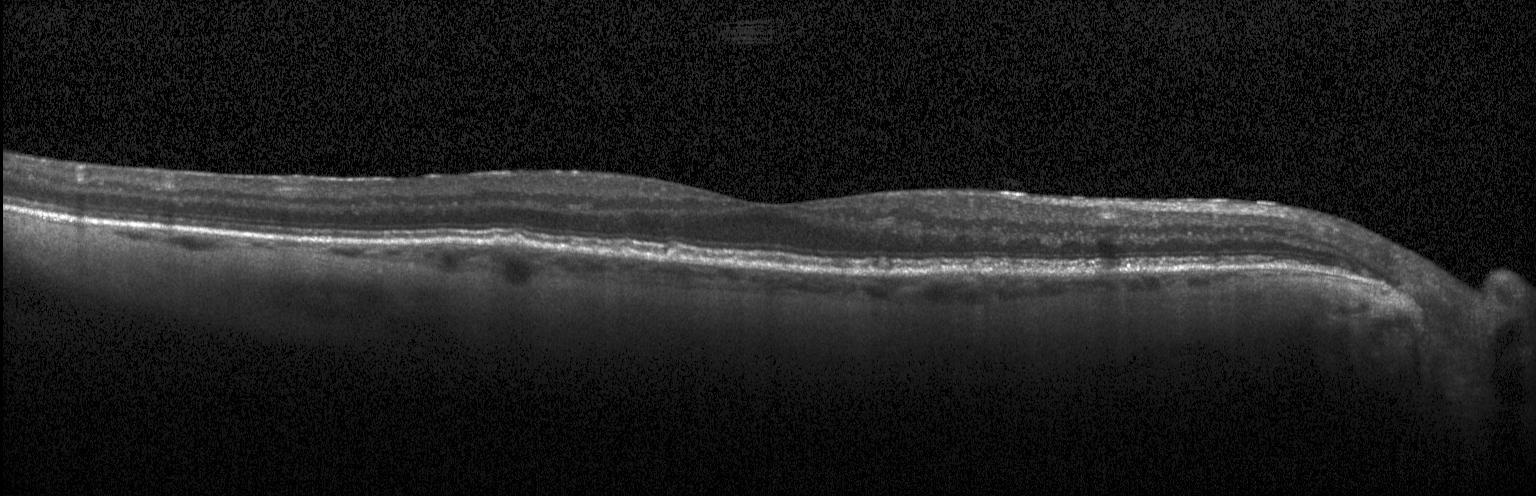 Heidelberg Spectralis OCT system · retinal OCT cross-section.
Multiple drusen.